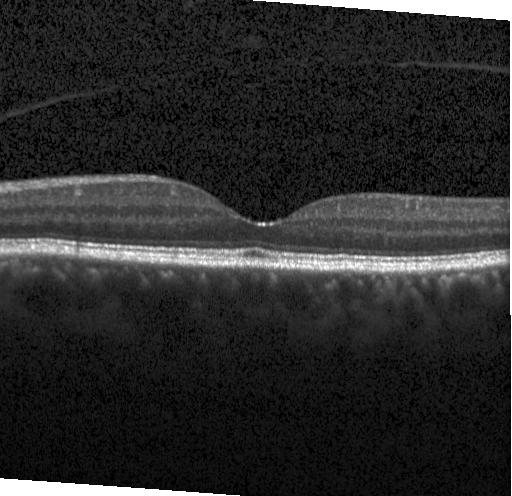 Heidelberg Spectralis · retinal OCT B-scan.
Macular OCT: no CNV, DME, or drusen.